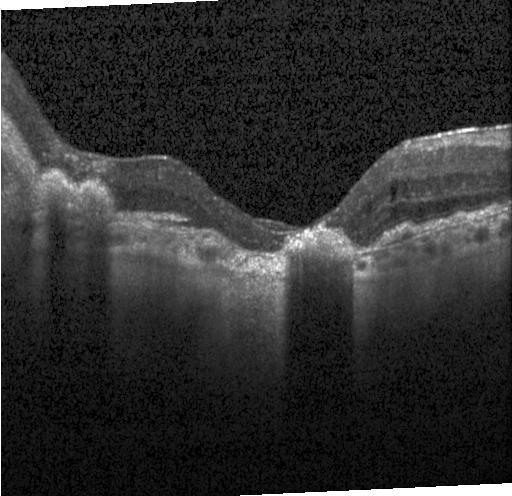

Macular scan, spectral-domain optical coherence tomography, OCT B-scan — OCT finding: a choroidal neovascular membrane.